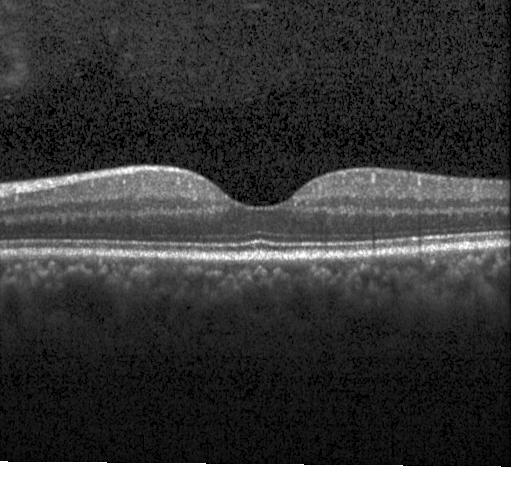
Spectral-domain OCT. Retinal OCT B-scan. Centered on the fovea. Heidelberg Spectralis OCT system — Dx: no evidence of choroidal neovascularization, diabetic macular edema, or drusen.